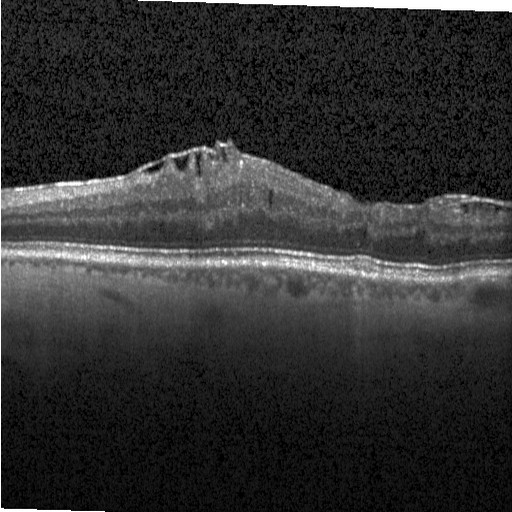

Assessment: diabetic macular edema.